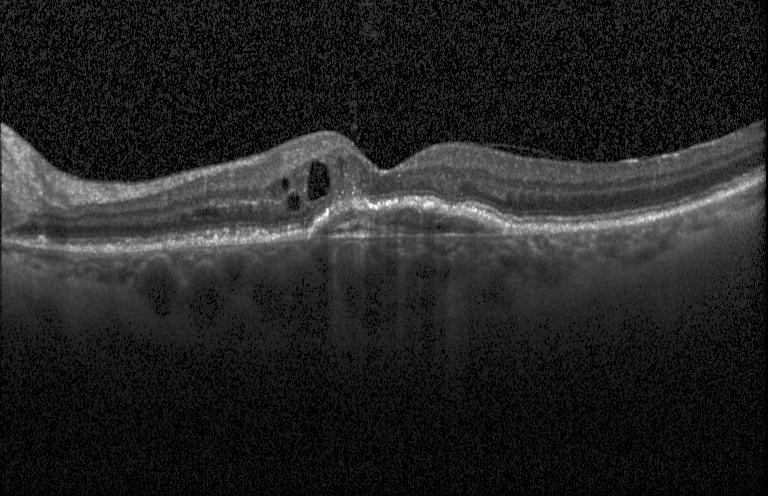
Retinal OCT B-scan. This B-scan demonstrates a choroidal neovascular membrane.